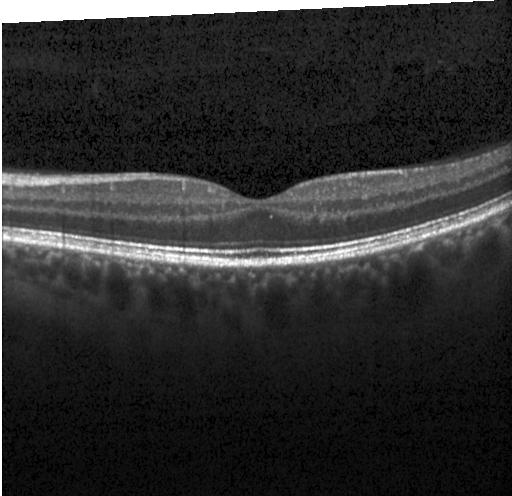 Macular OCT: neither choroidal neovascularization, diabetic macular edema, nor drusen.